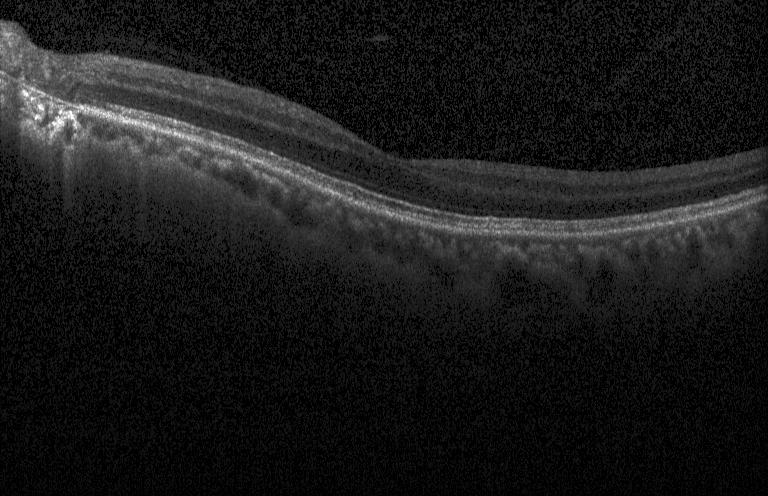

Macular OCT demonstrating no evidence of choroidal neovascularization, diabetic macular edema, or drusen.